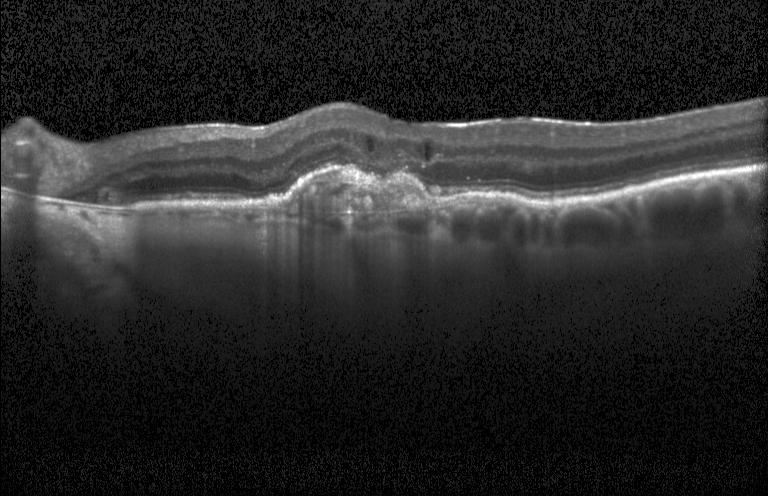
Optical coherence tomography scan; spectral-domain optical coherence tomography. Dx: CNV.